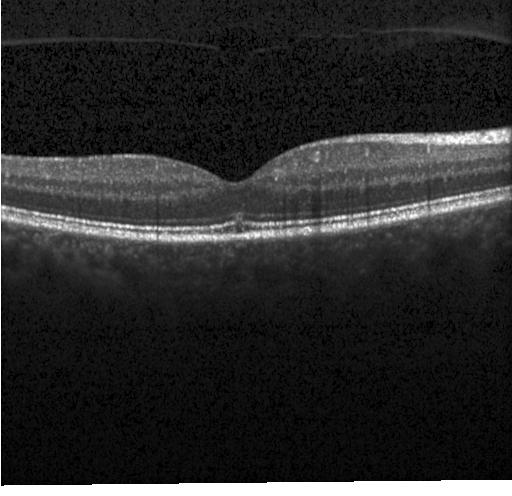
Retinal OCT cross-section showing neither choroidal neovascularization, diabetic macular edema, nor drusen.